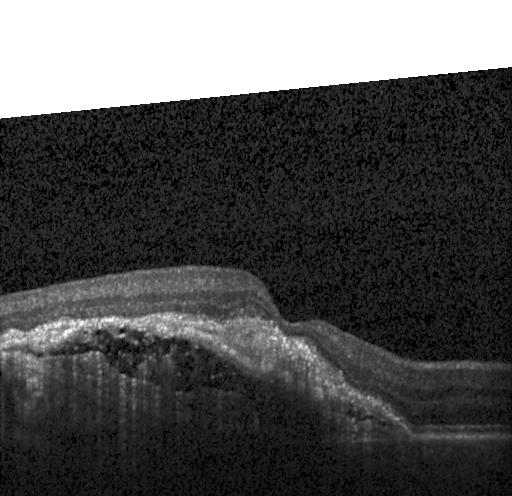
Retinal OCT B-scan — This B-scan demonstrates choroidal neovascularization.